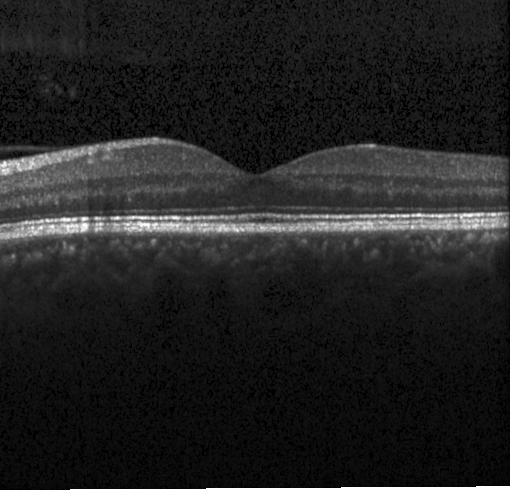 Diagnosis: neither choroidal neovascularization, diabetic macular edema, nor drusen.